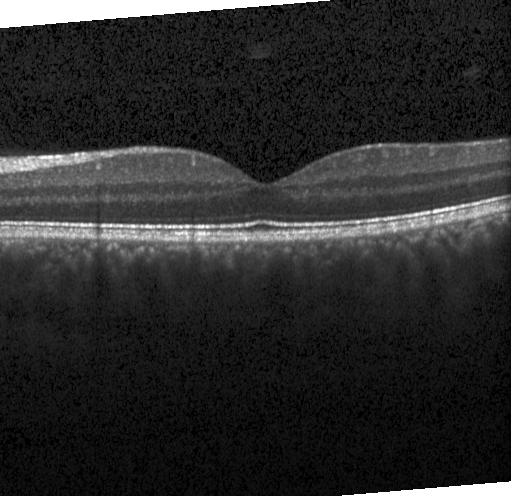
OCT scan showing no CNV, DME, or drusen.